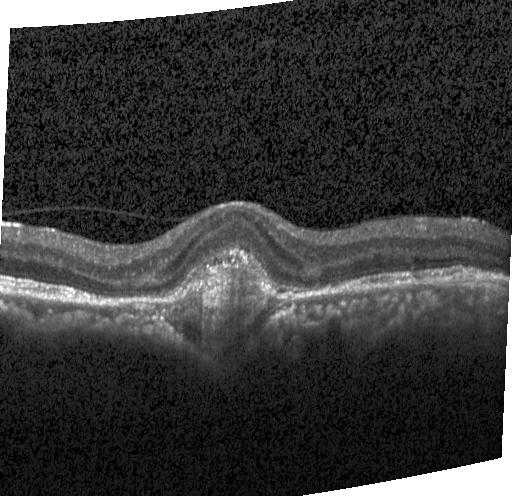

Retinal OCT cross-section showing choroidal neovascularization.